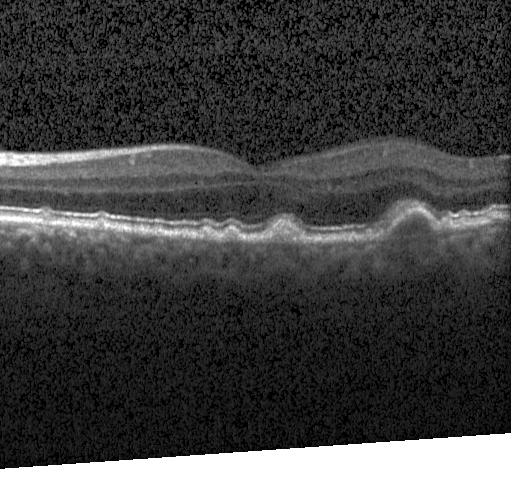
OCT scan showing sub-RPE drusenoid deposits.